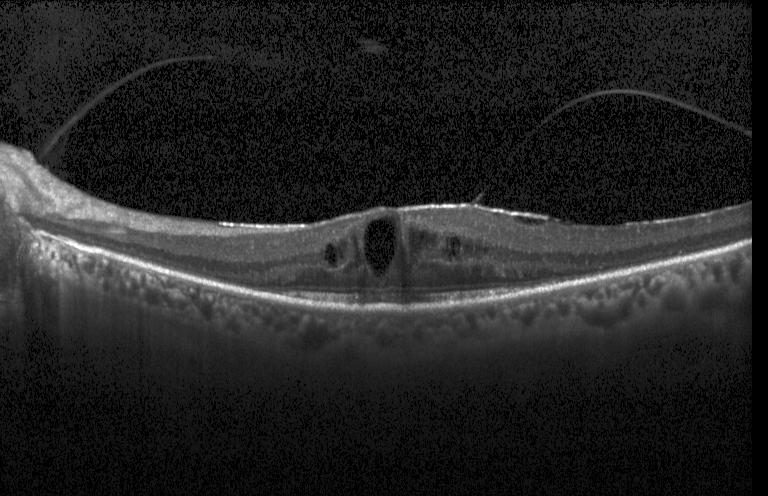 Assessment: diabetic macular edema.